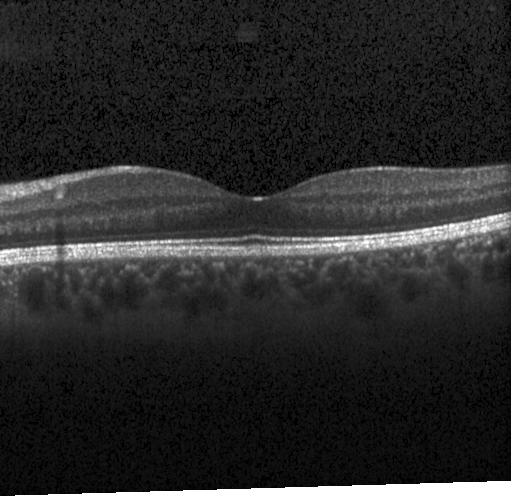 Finding: neither choroidal neovascularization, diabetic macular edema, nor drusen.